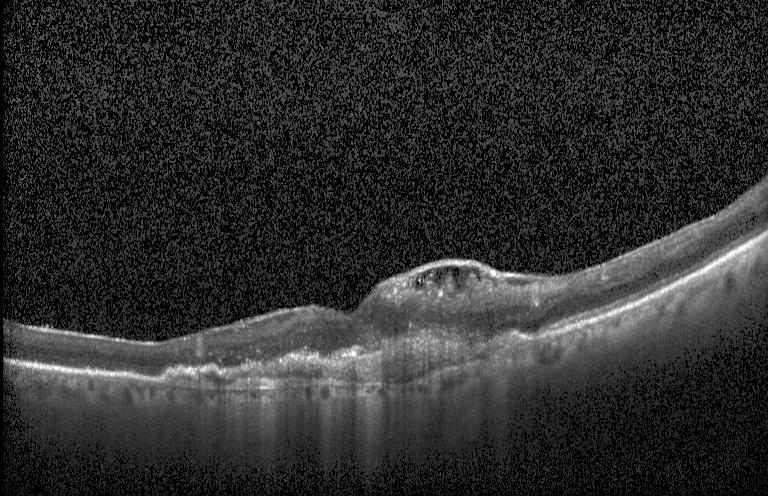 Spectral-domain OCT B-scan: choroidal neovascularization (CNV).